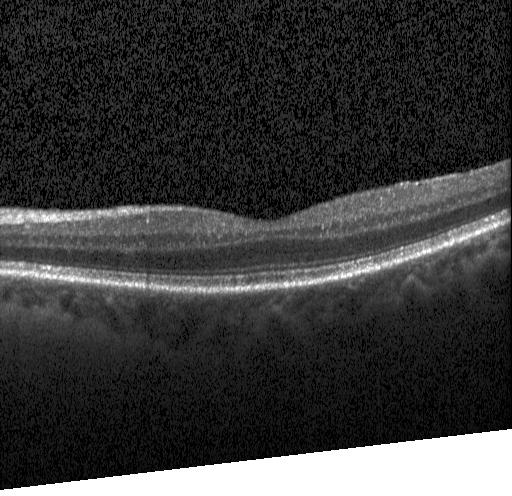

OCT finding: no CNV, no DME, and no drusen.